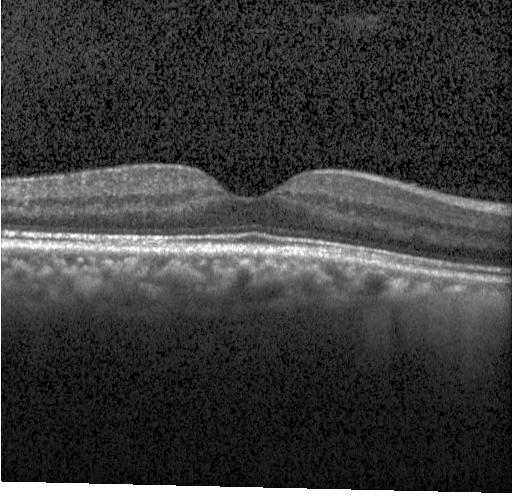

SD-OCT · retinal OCT cross-section · Heidelberg Spectralis · fovea-centered — OCT finding: no evidence of CNV, DME, or drusen.